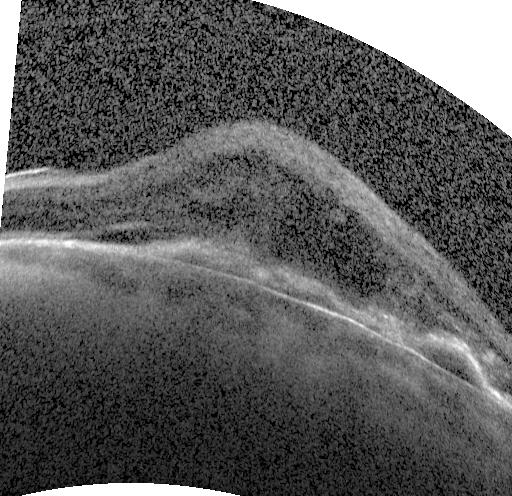

OCT finding: choroidal neovascularization.